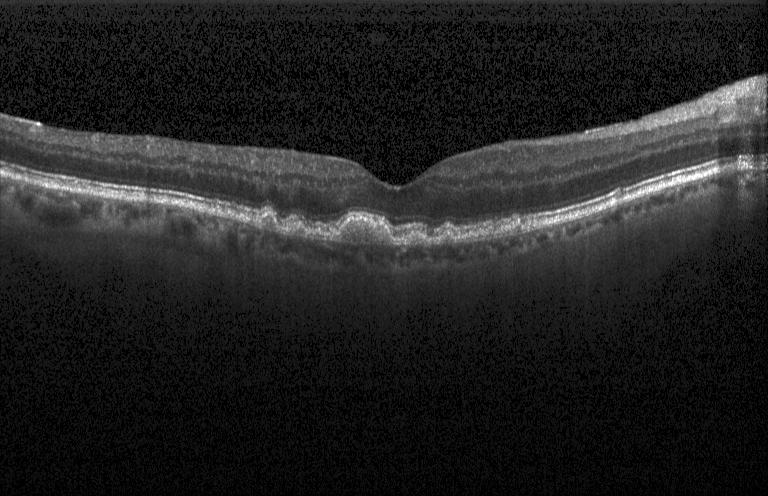 OCT line scan
Impression: sub-RPE drusenoid deposits.